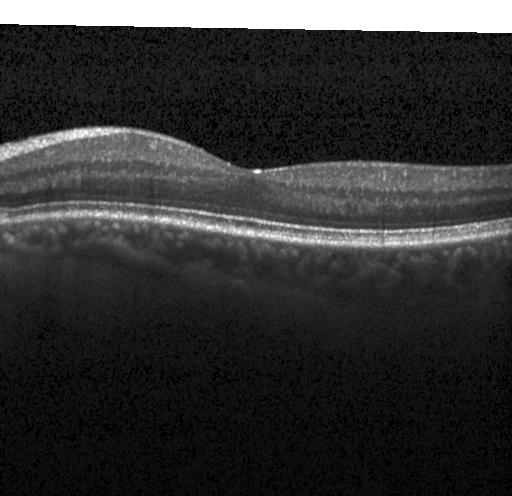 OCT line scan. Centered on the fovea. SD-OCT. OCT finding: no choroidal neovascularization, diabetic macular edema, or drusen.